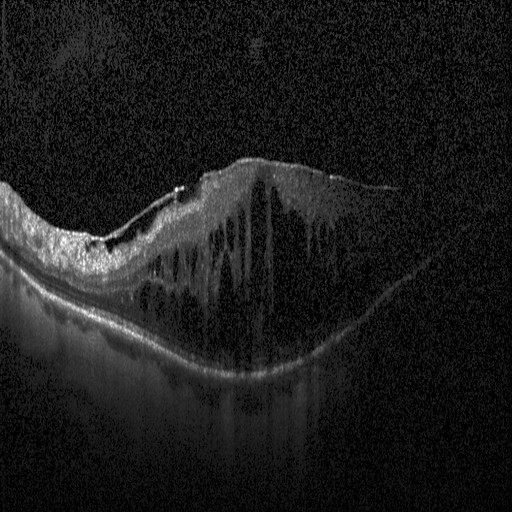 Heidelberg Spectralis OCT system, spectral-domain optical coherence tomography, optical coherence tomography B-scan, macular scan — Impression: diabetic macular edema (DME).